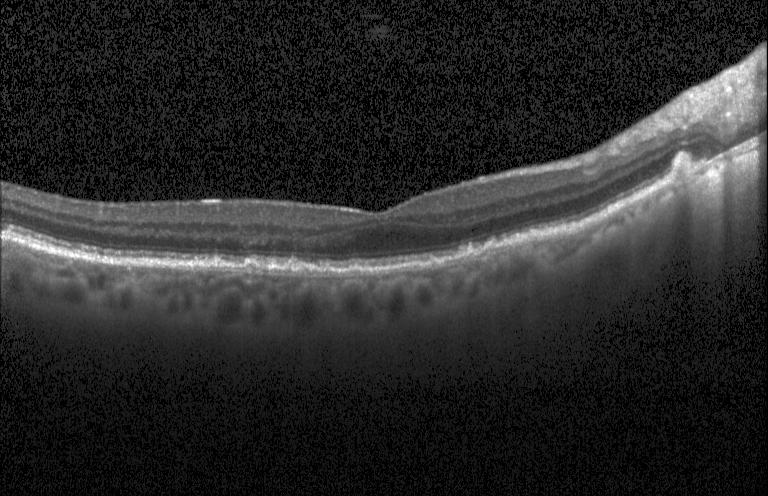
Centered on the fovea; retinal OCT B-scan
The scan shows drusen.